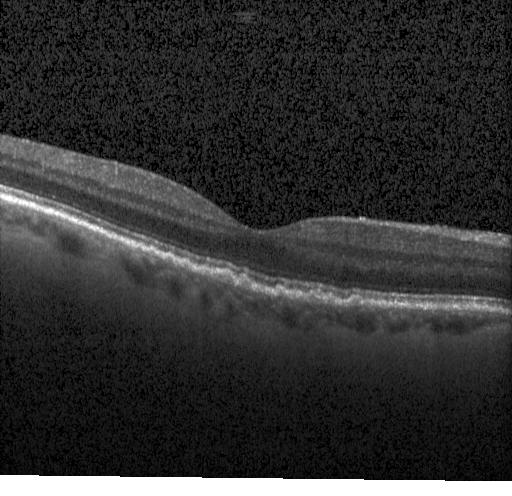 Macular OCT demonstrating multiple drusen.